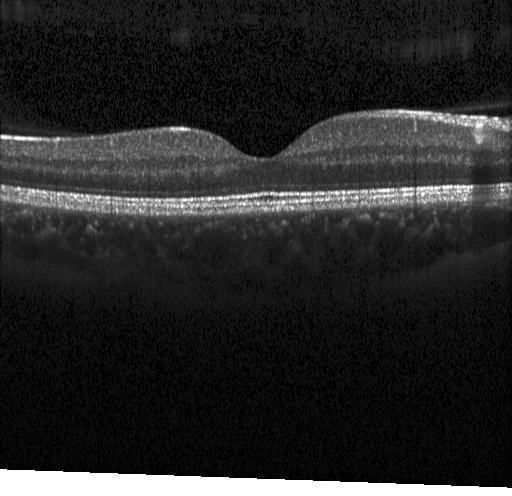
Impression: neither choroidal neovascularization, diabetic macular edema, nor drusen.